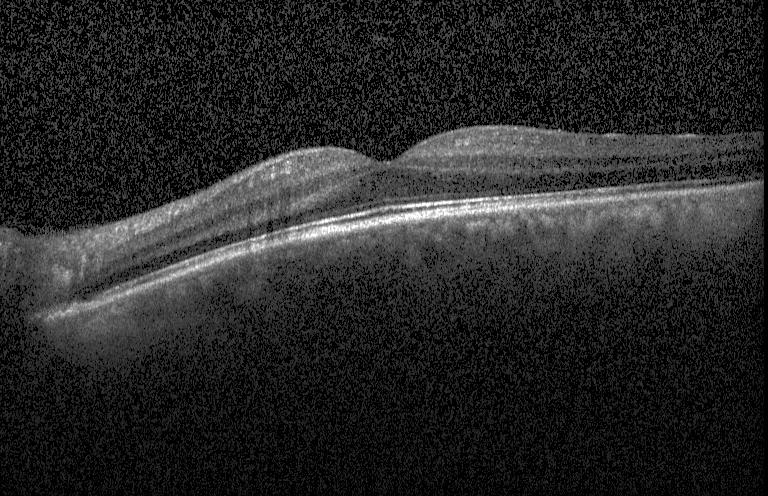

Retinal OCT B-scan — Neither CNV, DME, nor drusen.